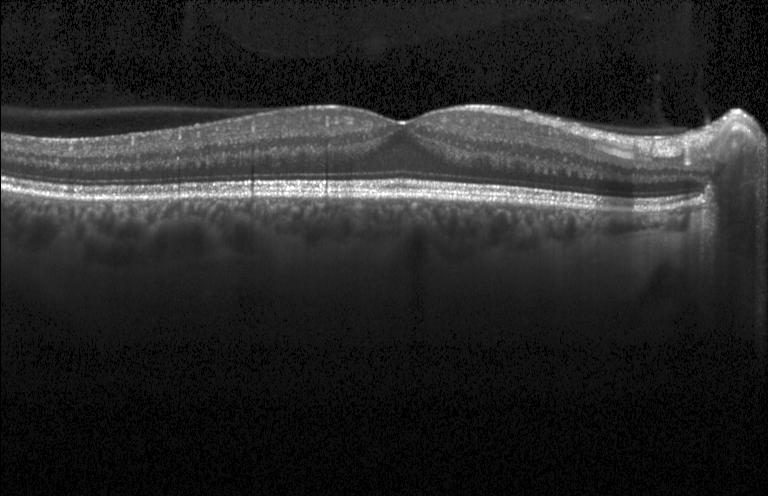
Diagnosis: no CNV, DME, or drusen.